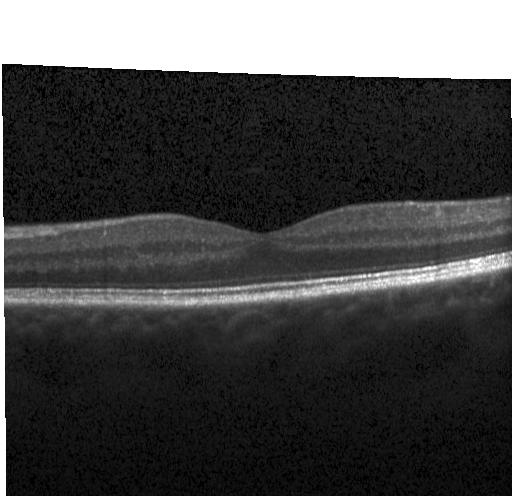 Retinal OCT B-scan · spectral-domain optical coherence tomography · Heidelberg Spectralis · macular scan. Macular OCT: neither choroidal neovascularization, diabetic macular edema, nor drusen.